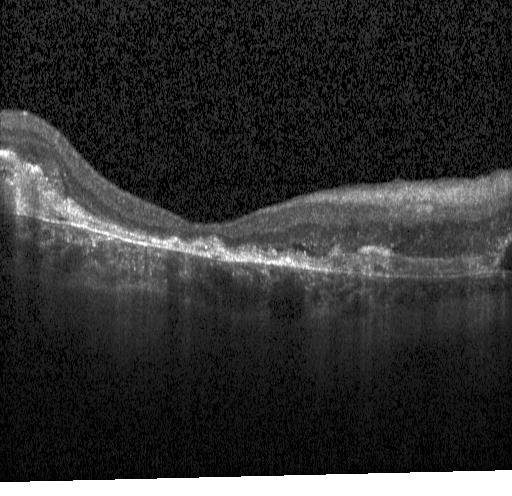
Retinal OCT cross-section
Diagnosis: a choroidal neovascular membrane.